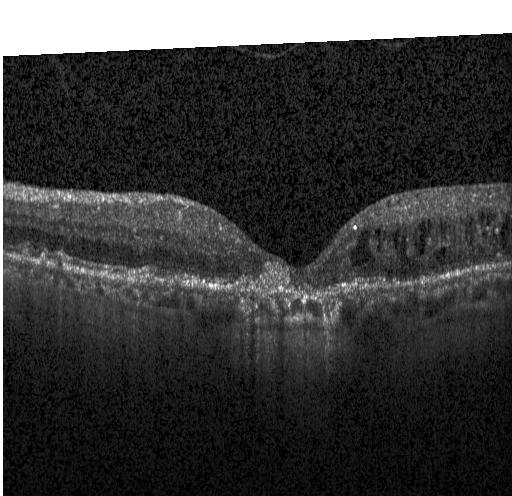 OCT scan showing choroidal neovascularization.